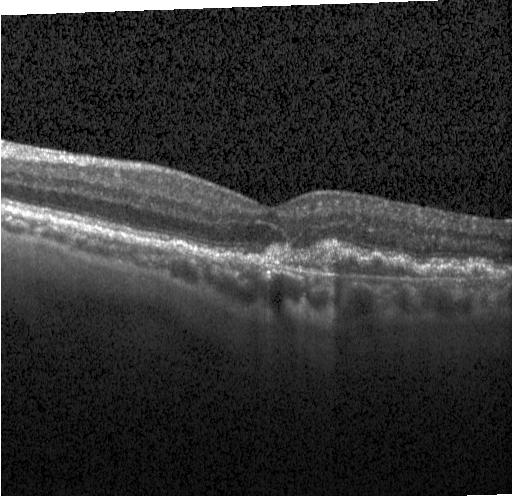
Retinal OCT B-scan · Heidelberg Spectralis · horizontal scan through the fovea.
Dx: choroidal neovascularization (CNV).